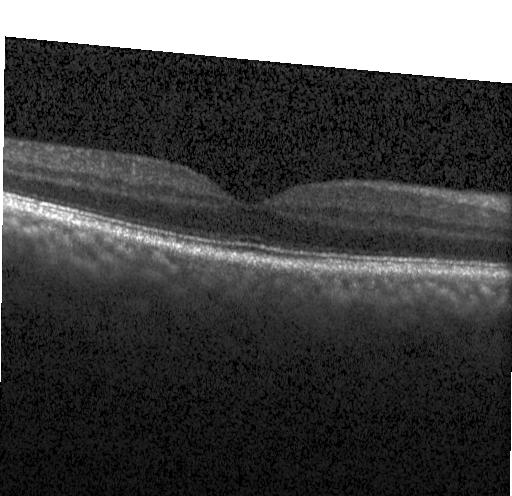

Diagnosis: neither choroidal neovascularization, diabetic macular edema, nor drusen.